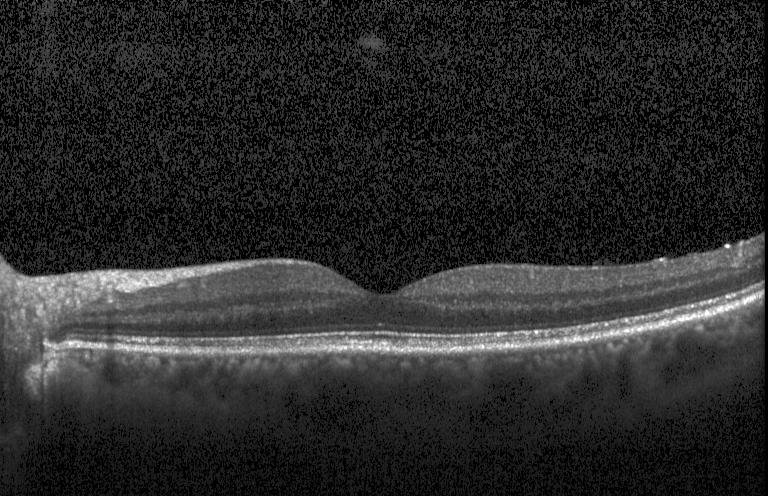 Diagnosis: neither choroidal neovascularization, diabetic macular edema, nor drusen.